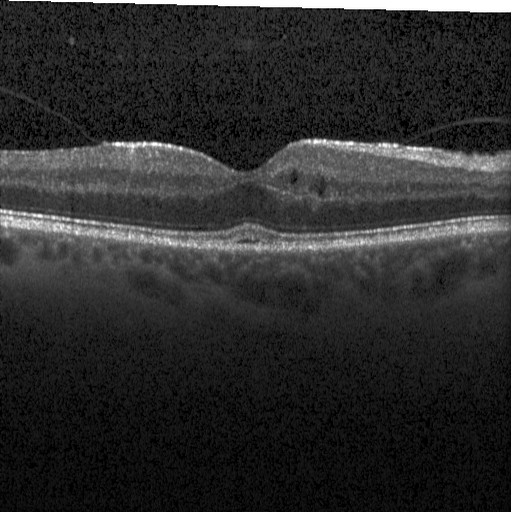

OCT B-scan — Impression: DME.